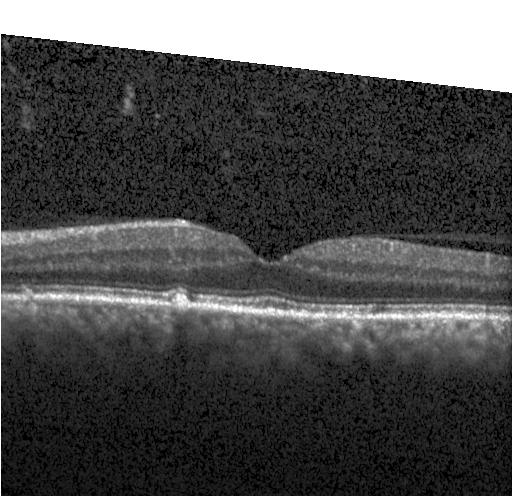

SD-OCT; optical coherence tomography scan
Macular OCT: multiple drusen.